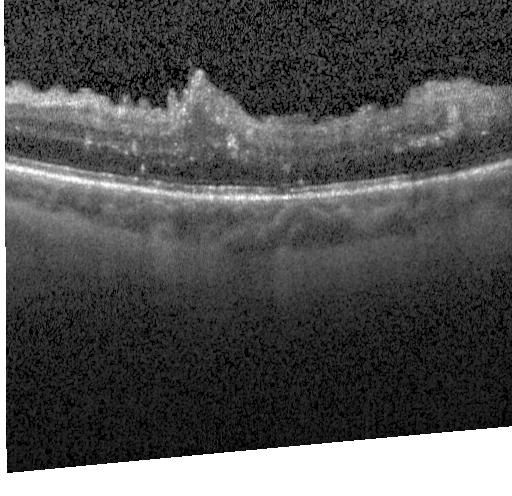
Retinal OCT B-scan — Assessment: DME.